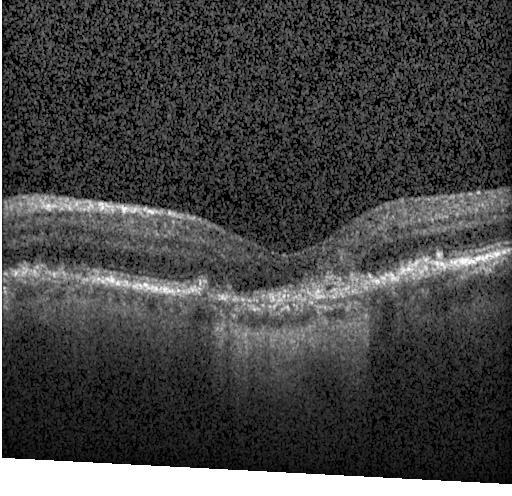 Optical coherence tomography B-scan. Heidelberg Spectralis. Spectral-domain OCT.
Diagnosis: choroidal neovascularization (CNV).